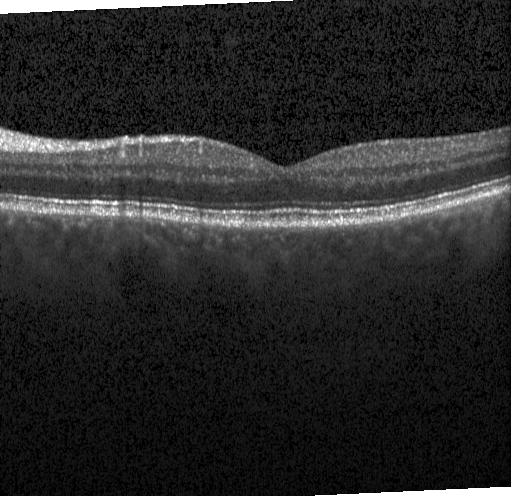

Spectral-domain OCT, optical coherence tomography B-scan, fovea-centered, instrument: Heidelberg Spectralis — This B-scan demonstrates no choroidal neovascularization, diabetic macular edema, or drusen.